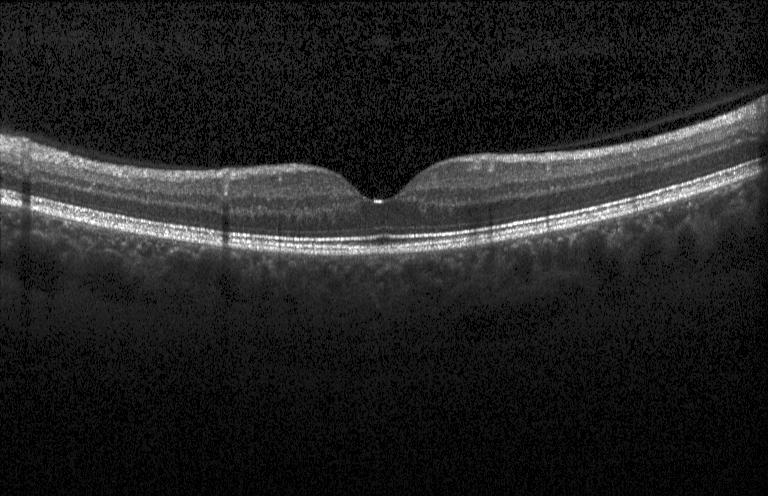

OCT finding: neither choroidal neovascularization, diabetic macular edema, nor drusen.